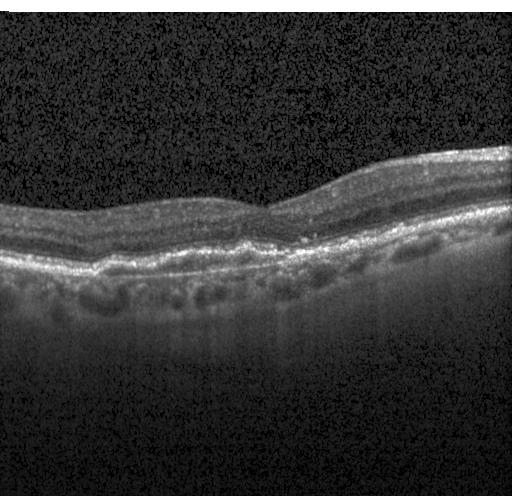 Acquired on a Heidelberg Spectralis, OCT line scan.
Assessment: a choroidal neovascular membrane.